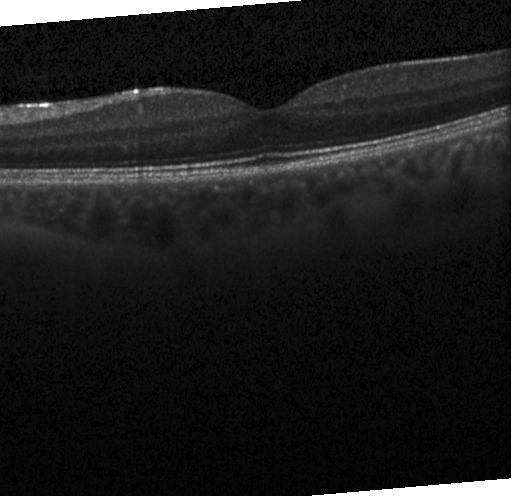

OCT line scan — This B-scan demonstrates neither CNV, DME, nor drusen.